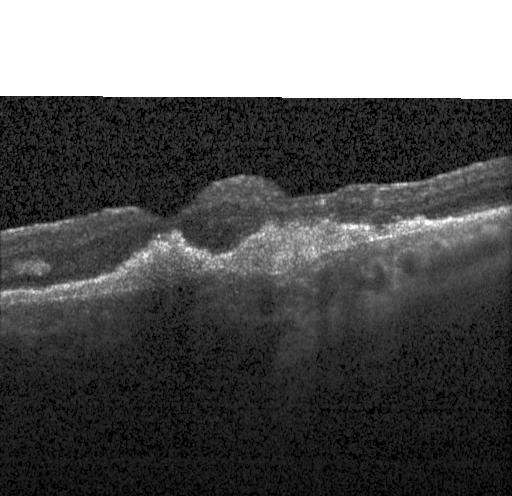 Heidelberg Spectralis, optical coherence tomography scan, centered on the fovea, spectral-domain optical coherence tomography — Impression: a choroidal neovascular membrane.